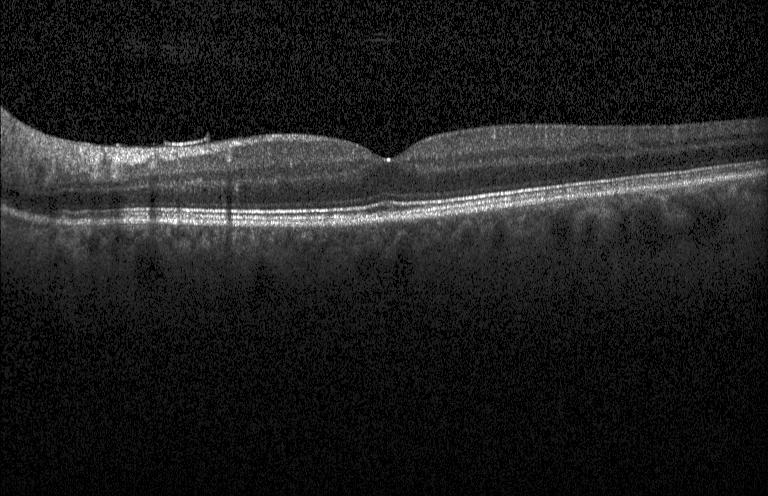 Spectral-domain OCT B-scan: no evidence of choroidal neovascularization, diabetic macular edema, or drusen.